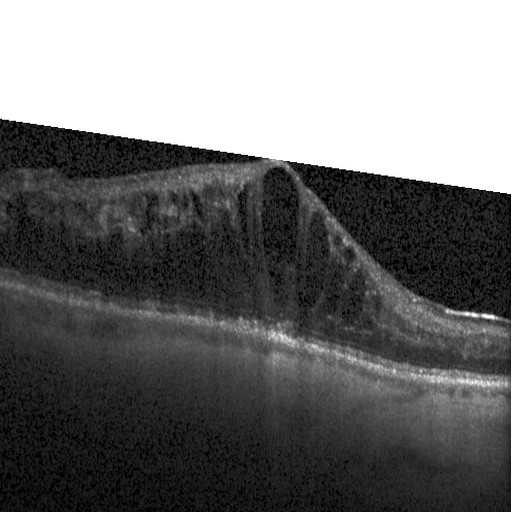
Retinal OCT cross-section.
OCT finding: DME.